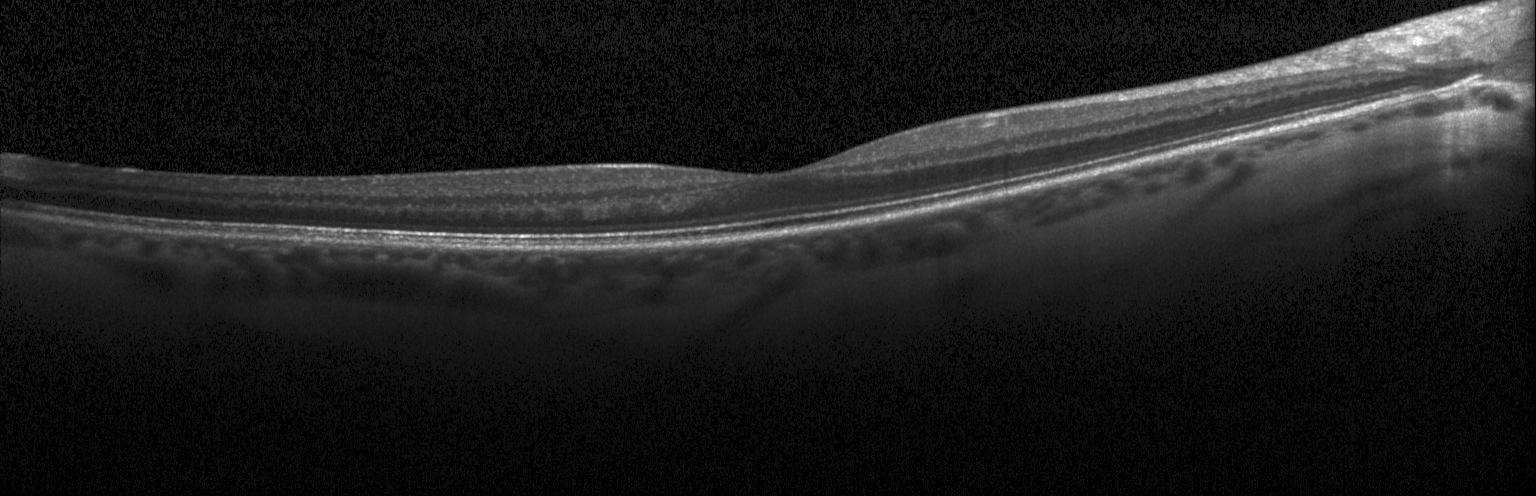 Impression: neither choroidal neovascularization, diabetic macular edema, nor drusen.